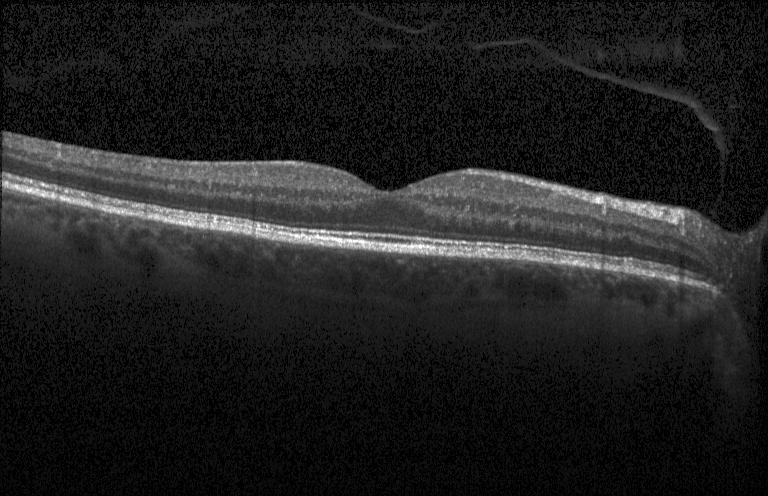 OCT B-scan, Heidelberg Spectralis OCT system, horizontal scan through the fovea — Impression: no choroidal neovascularization, no diabetic macular edema, and no drusen.